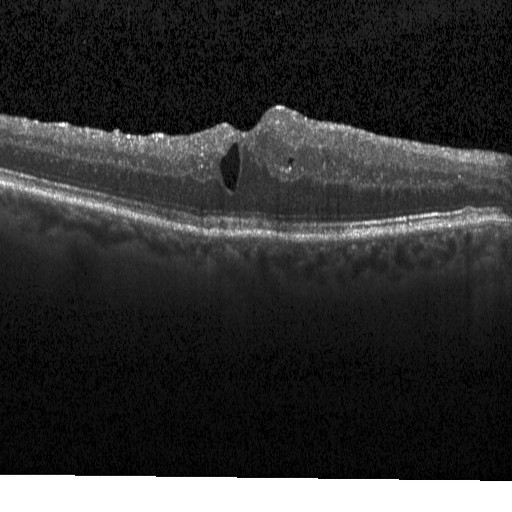 This B-scan demonstrates diabetic macular edema (DME).